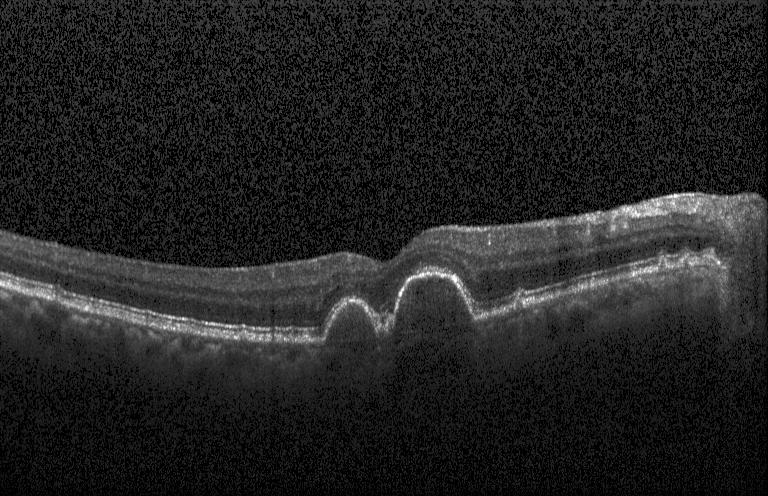
Spectral-domain OCT. Heidelberg Spectralis. Retinal OCT cross-section. Through the macula — Impression: drusen.